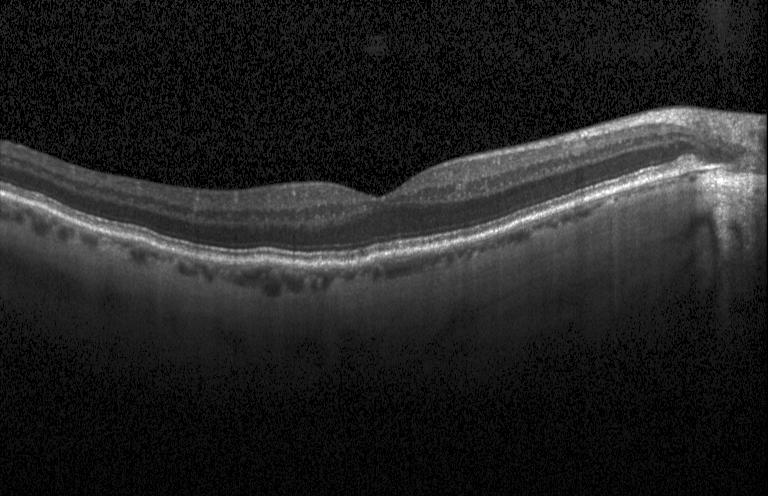 Retinal OCT cross-section · horizontal scan through the fovea. No CNV, no DME, and no drusen.